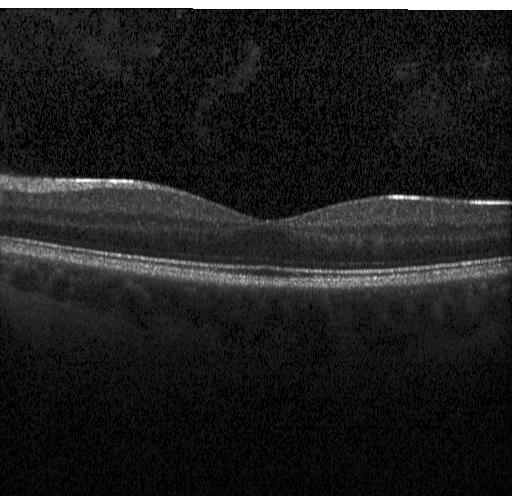 OCT line scan — The scan shows no choroidal neovascularization, no diabetic macular edema, and no drusen.